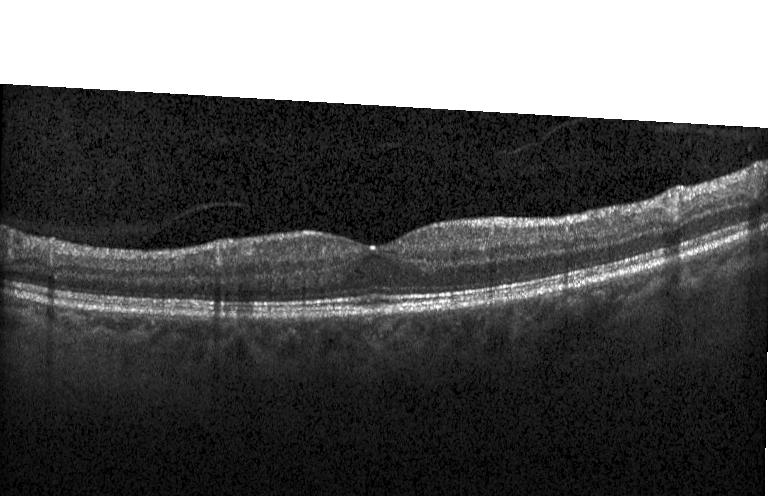
Impression: no CNV, DME, or drusen.